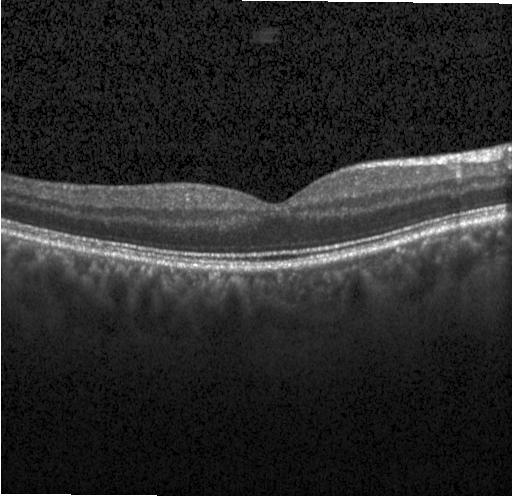
Assessment: neither choroidal neovascularization, diabetic macular edema, nor drusen.